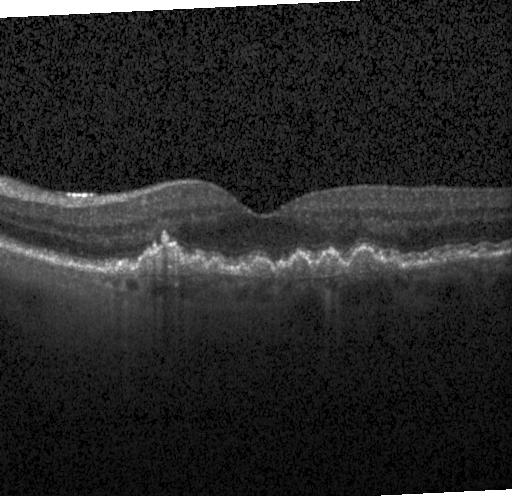
Retinal OCT B-scan — The scan shows sub-RPE drusenoid deposits.